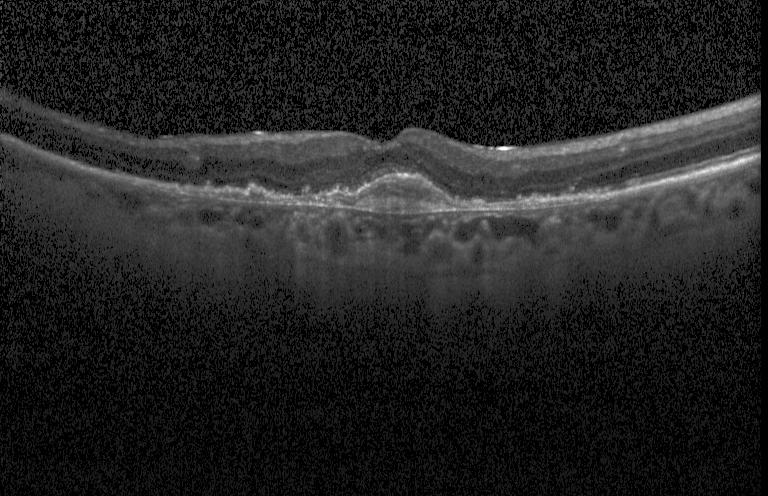 OCT B-scan.
Assessment: a choroidal neovascular membrane.